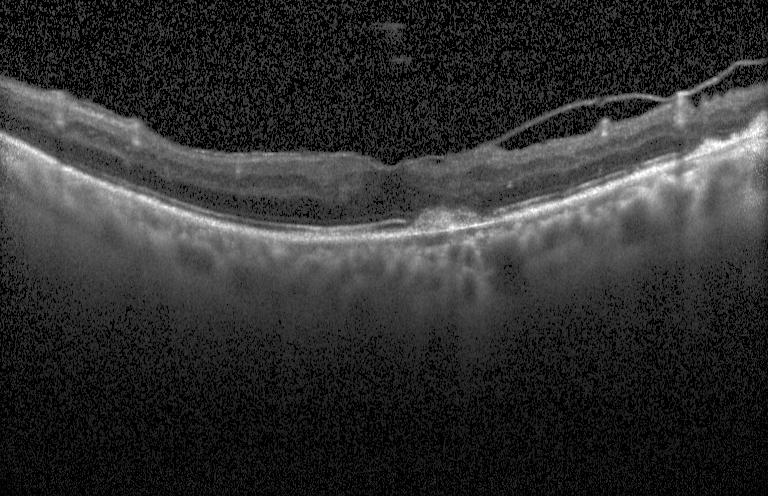 OCT line scan
Impression: choroidal neovascularization (CNV).